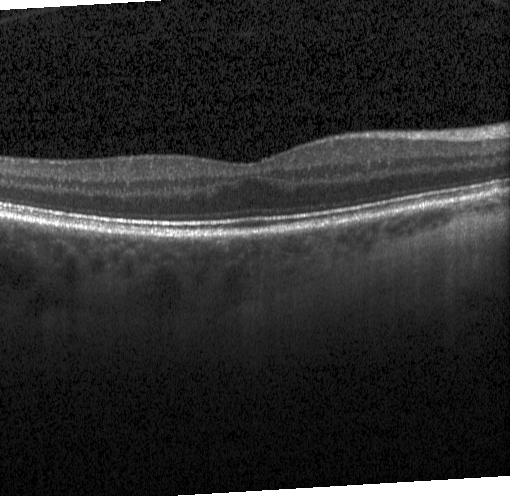
Spectral-domain optical coherence tomography, OCT line scan, instrument: Heidelberg Spectralis, horizontal scan through the fovea
Impression: neither CNV, DME, nor drusen.